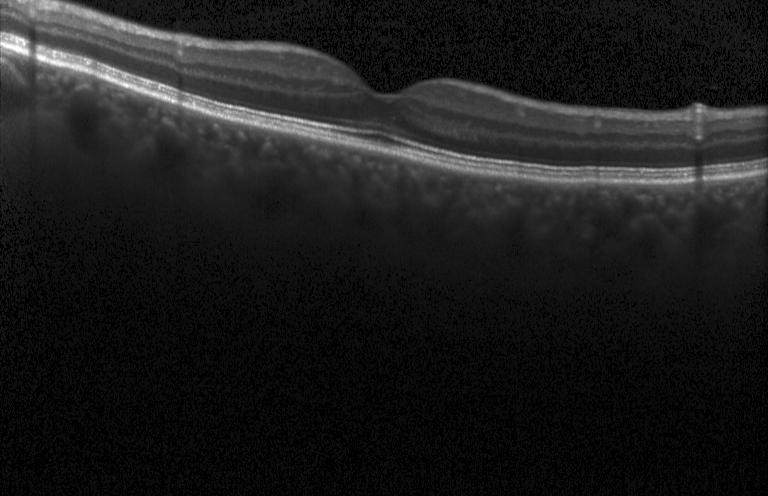
OCT B-scan. Spectral-domain optical coherence tomography. Macular scan. Heidelberg Spectralis.
Diagnosis: no evidence of CNV, DME, or drusen.